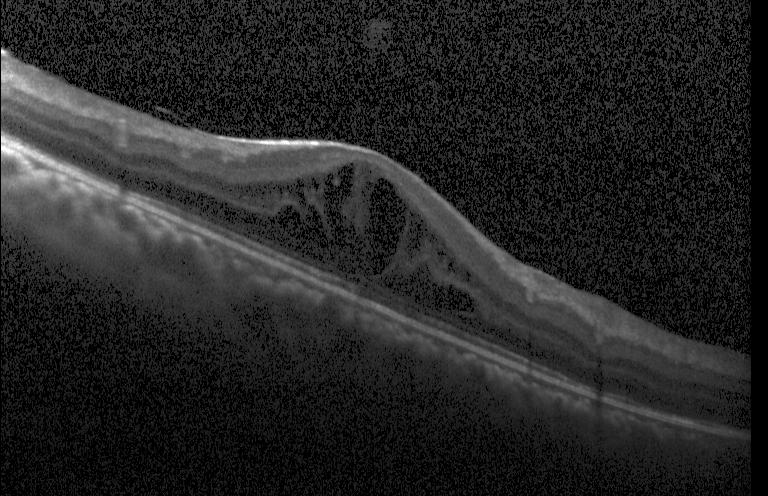 Macular OCT: diabetic macular edema (DME).